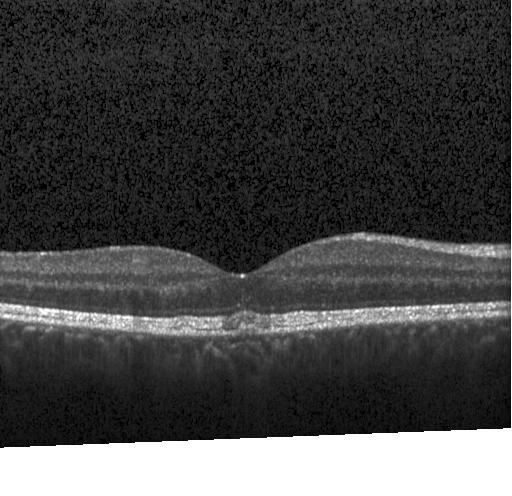

Spectral-domain OCT · Heidelberg Spectralis · optical coherence tomography B-scan. Dx: multiple drusen.